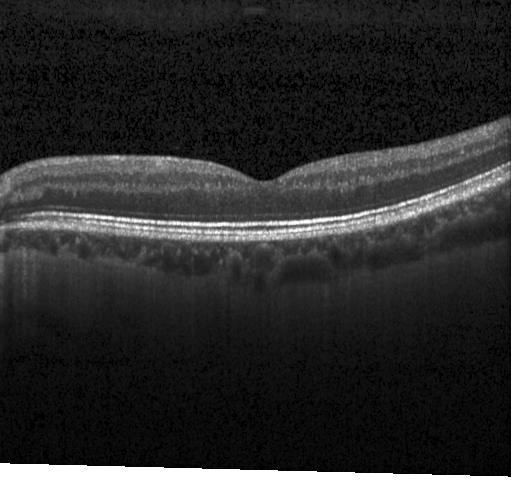
Centered on the fovea; OCT line scan
Impression: no choroidal neovascularization, no diabetic macular edema, and no drusen.